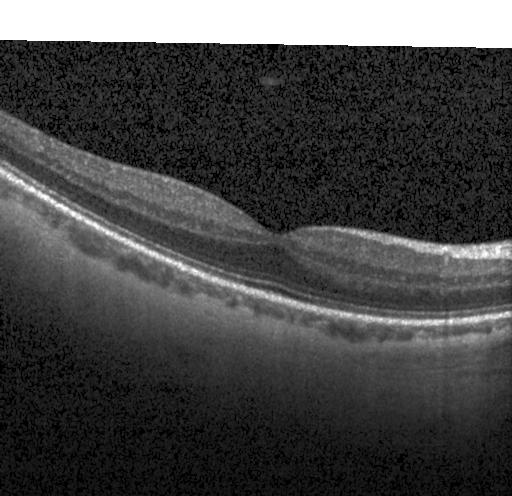 Through the macula · spectral-domain optical coherence tomography · acquired on a Heidelberg Spectralis · retinal OCT cross-section — Macular OCT: no choroidal neovascularization, diabetic macular edema, or drusen.